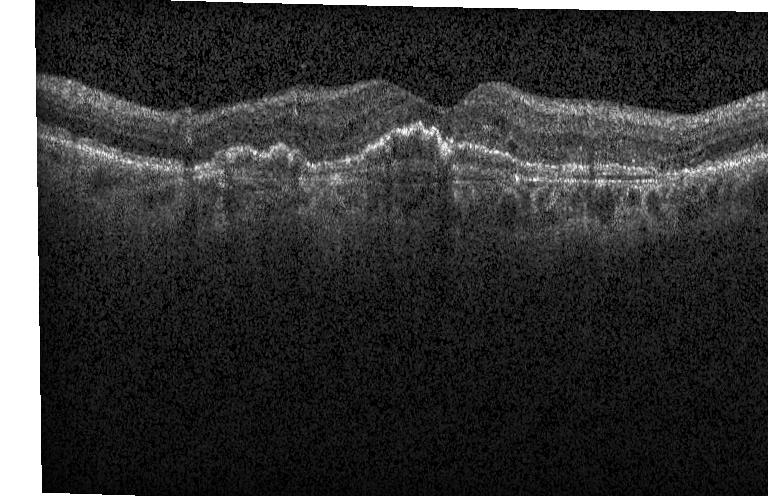 OCT B-scan, acquired on a Heidelberg Spectralis.
Impression: choroidal neovascularization.